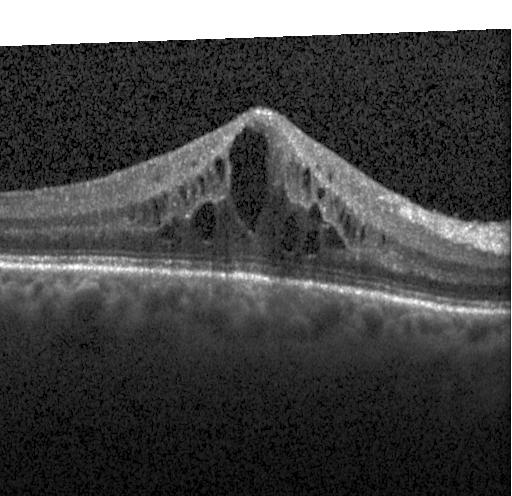 Finding: diabetic macular edema (DME).